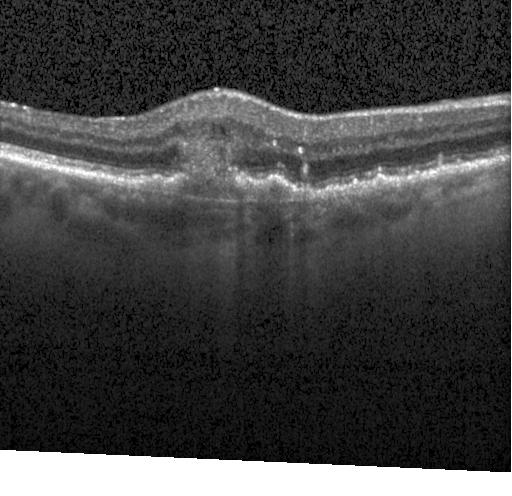
Instrument: Heidelberg Spectralis. Through the macula. OCT line scan. Spectral-domain OCT
Finding: a choroidal neovascular membrane.